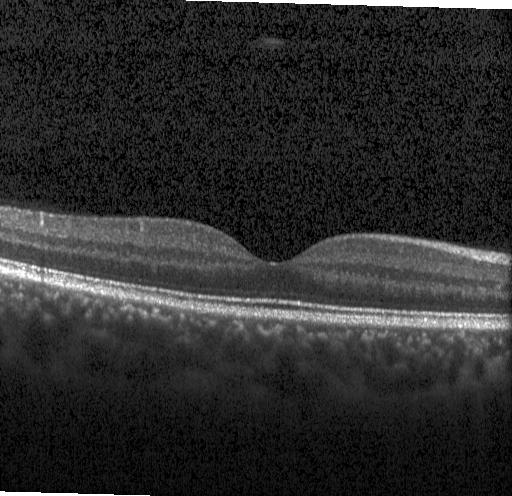 Retinal OCT B-scan; SD-OCT; acquired on a Heidelberg Spectralis; centered on the fovea
Dx: no evidence of choroidal neovascularization, diabetic macular edema, or drusen.